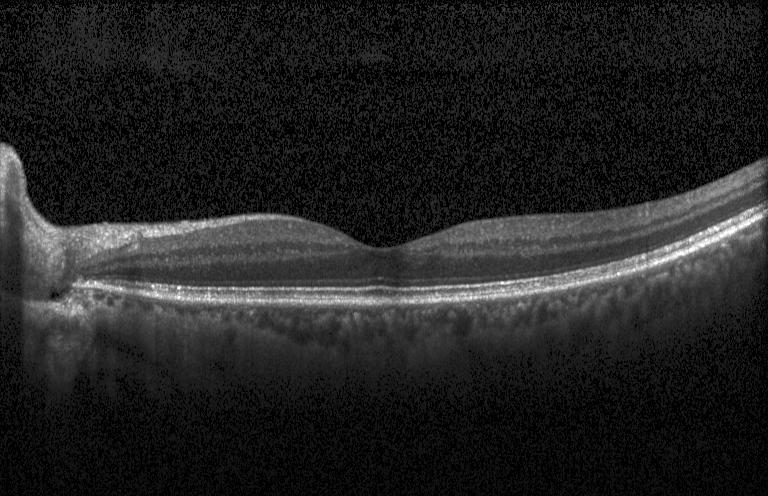

Spectral-domain optical coherence tomography; optical coherence tomography B-scan; through the macula — No evidence of choroidal neovascularization, diabetic macular edema, or drusen.